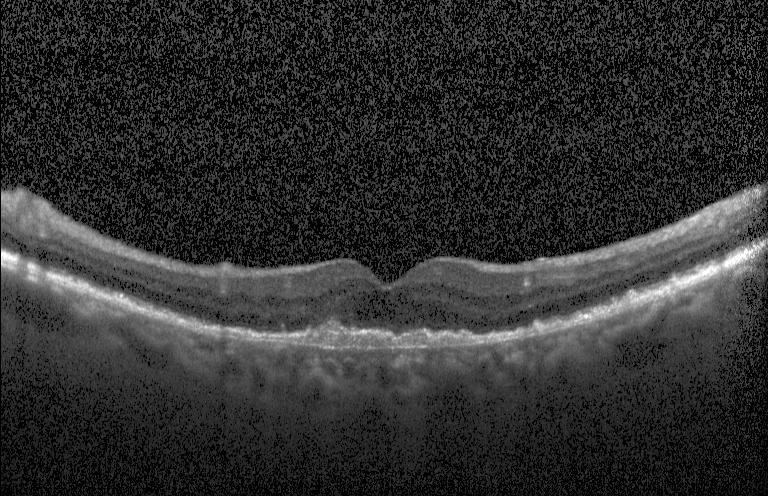

Macular OCT: a choroidal neovascular membrane.